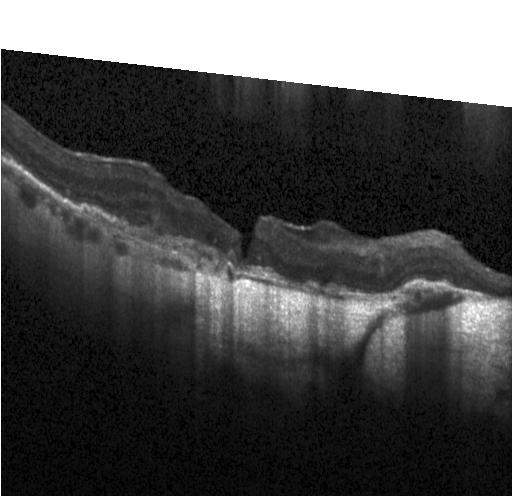 Macular OCT demonstrating a choroidal neovascular membrane.